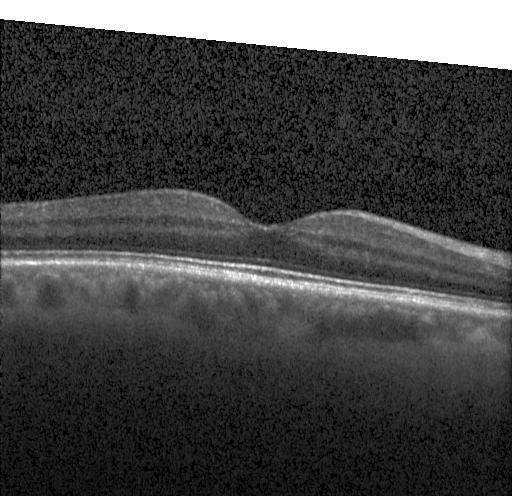

OCT line scan. Instrument: Heidelberg Spectralis. Horizontal scan through the fovea — Impression: no evidence of choroidal neovascularization, diabetic macular edema, or drusen.